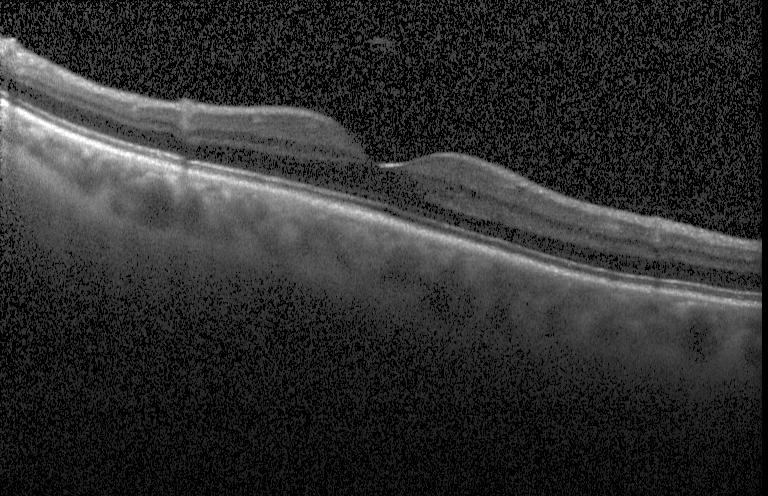
Acquired on a Heidelberg Spectralis; OCT line scan; spectral-domain OCT; fovea-centered — Macular OCT: no evidence of CNV, DME, or drusen.